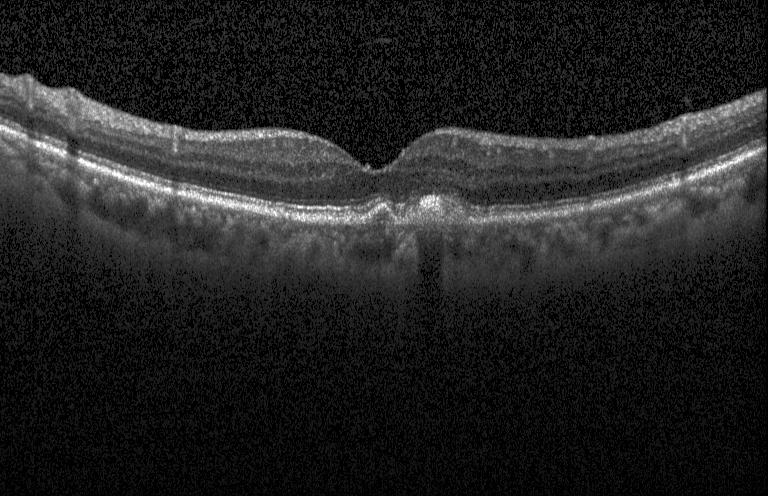
Horizontal scan through the fovea · OCT B-scan — Impression: sub-RPE drusenoid deposits.